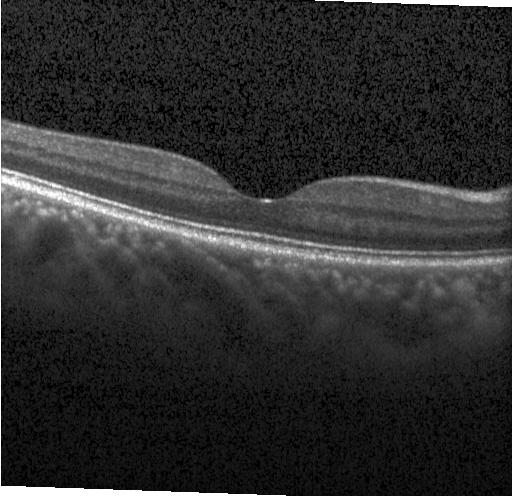
Finding: no CNV, DME, or drusen.